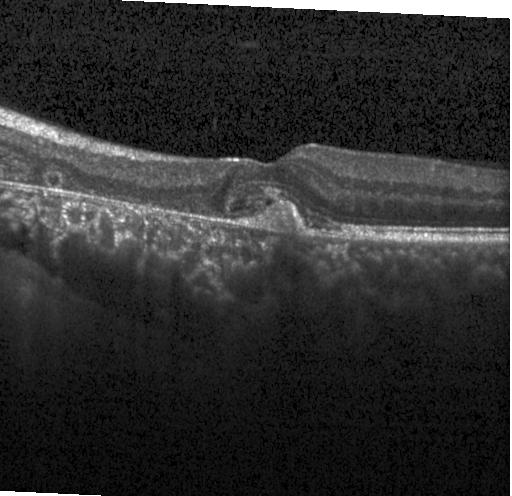 Retinal OCT cross-section, spectral-domain OCT, acquired on a Heidelberg Spectralis — Assessment: choroidal neovascularization (CNV).